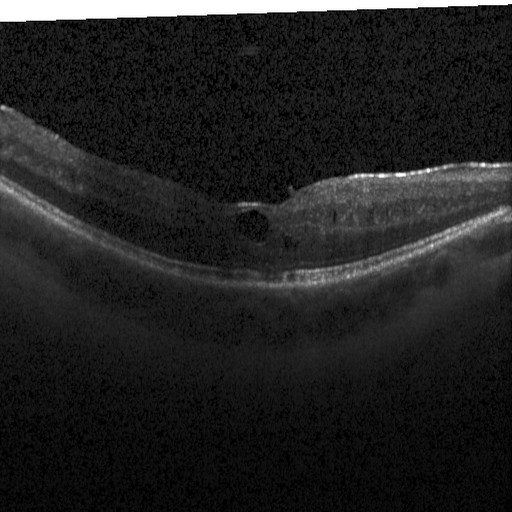 Retinal OCT B-scan. The scan shows diabetic macular edema (DME).